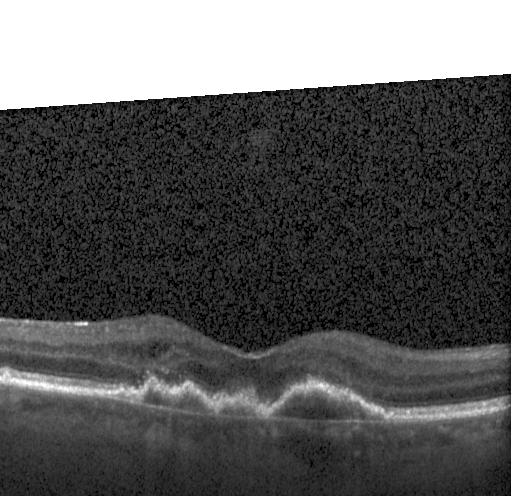 Retinal OCT B-scan. Spectral-domain optical coherence tomography. Macular scan.
Finding: a choroidal neovascular membrane.